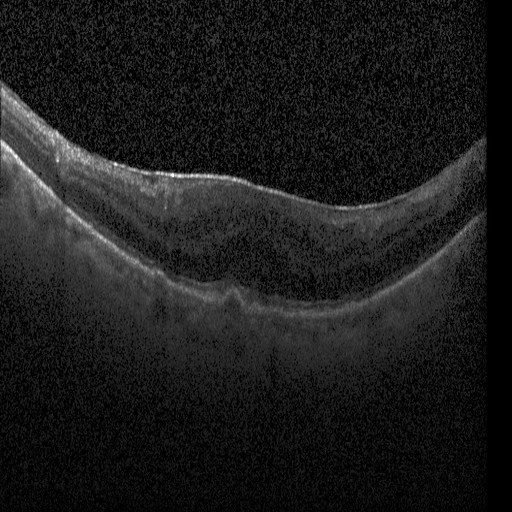

Diagnosis: diabetic macular edema (DME).